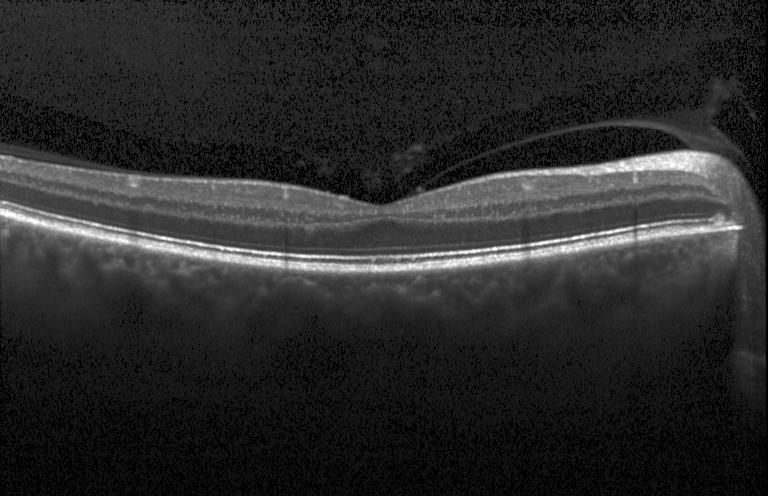 Finding: no choroidal neovascularization, diabetic macular edema, or drusen.